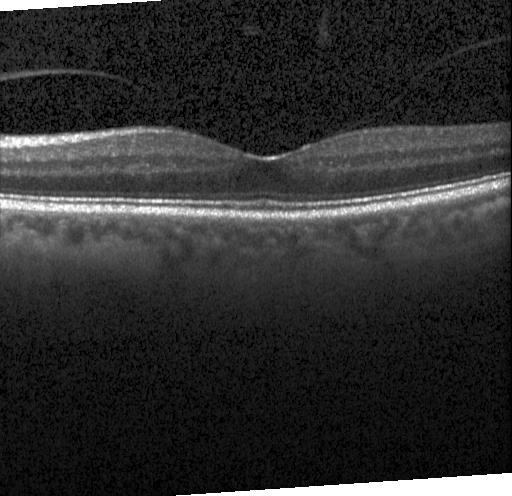 Finding: no choroidal neovascularization, diabetic macular edema, or drusen.